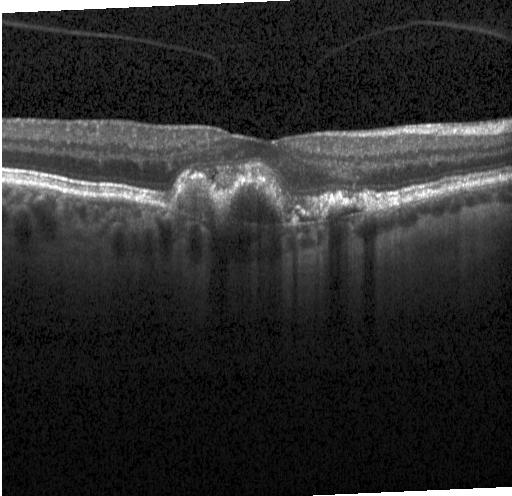
Optical coherence tomography B-scan.
Finding: a choroidal neovascular membrane.